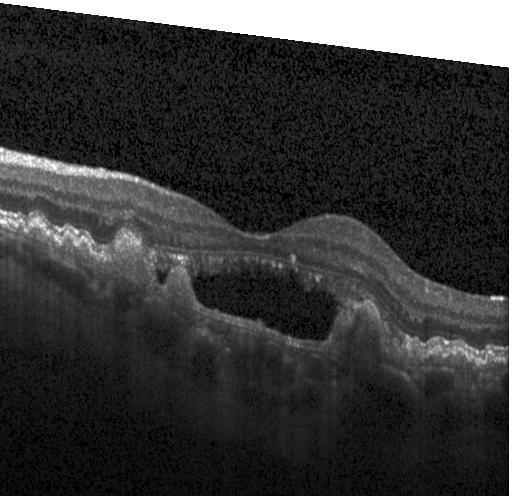

Finding: CNV.